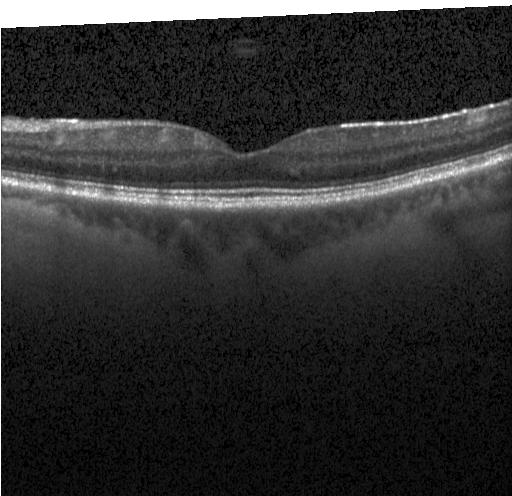

Heidelberg Spectralis OCT system; fovea-centered; optical coherence tomography scan; spectral-domain OCT — Impression: neither CNV, DME, nor drusen.